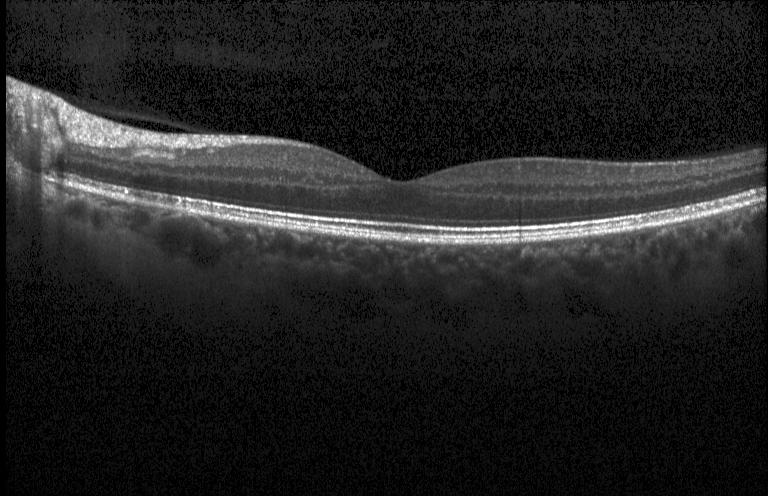

Optical coherence tomography scan, through the macula, spectral-domain optical coherence tomography
Finding: no CNV, DME, or drusen.